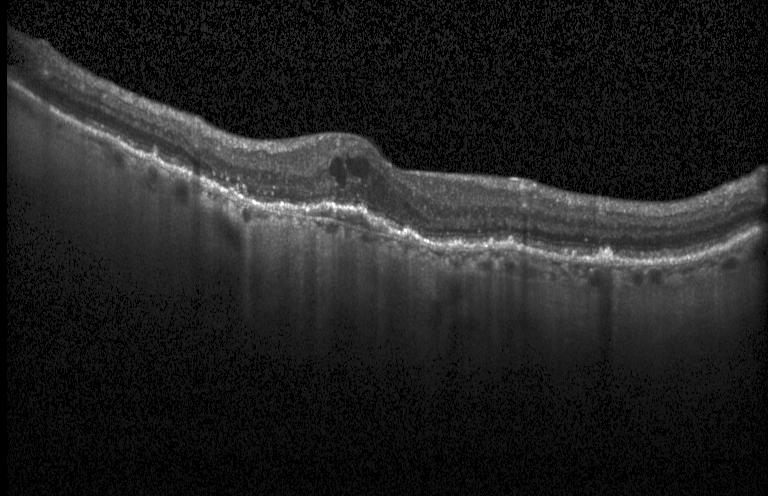 OCT B-scan · SD-OCT. Impression: choroidal neovascularization (CNV).